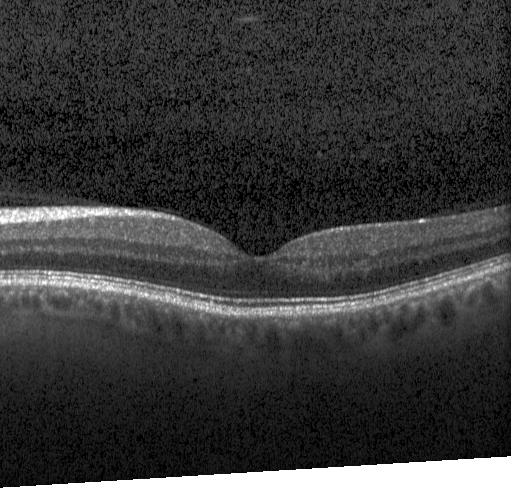 Instrument: Heidelberg Spectralis; spectral-domain OCT; retinal OCT B-scan; through the macula. OCT finding: no choroidal neovascularization, no diabetic macular edema, and no drusen.